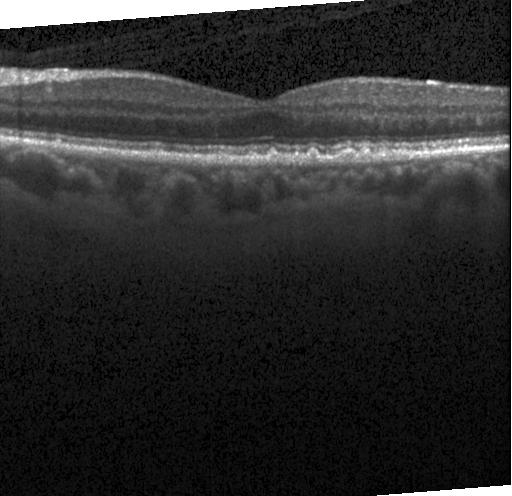
Impression: drusen.